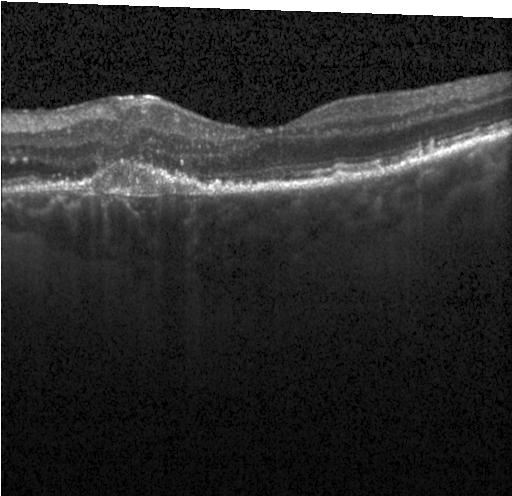 Dx: choroidal neovascularization.